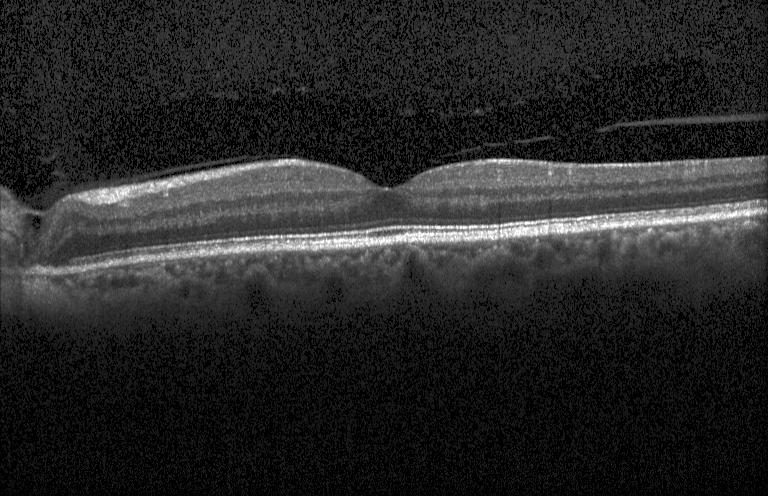 Retinal OCT B-scan; instrument: Heidelberg Spectralis — This B-scan demonstrates no choroidal neovascularization, diabetic macular edema, or drusen.